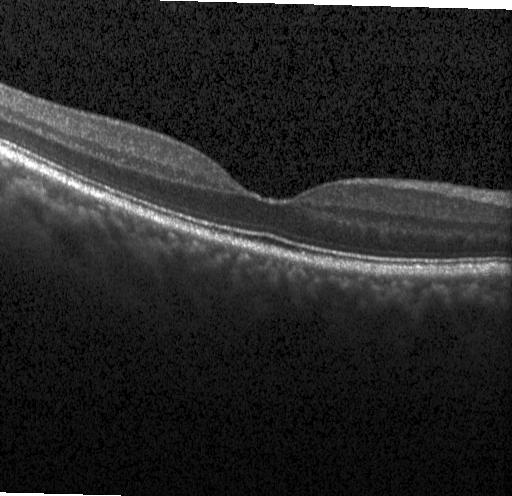 Fovea-centered · OCT B-scan · SD-OCT · Heidelberg Spectralis OCT system
OCT finding: no choroidal neovascularization, diabetic macular edema, or drusen.